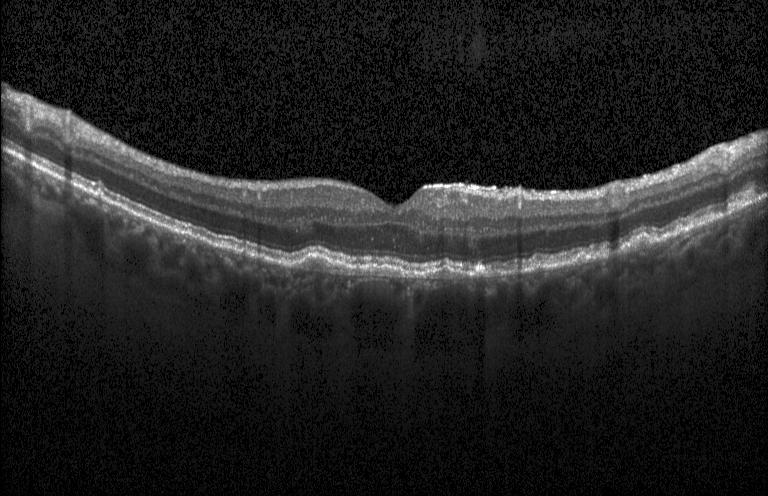 Macular OCT: a choroidal neovascular membrane.